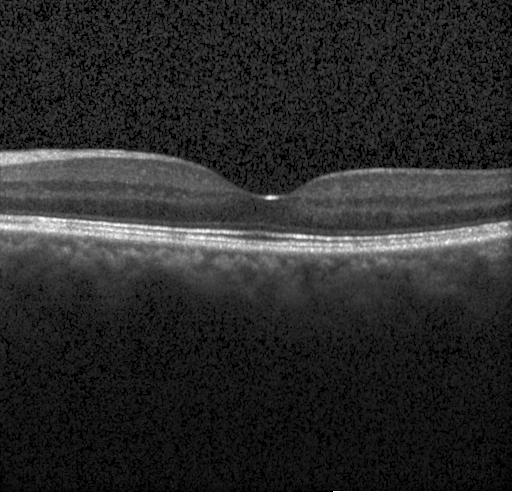 Horizontal scan through the fovea. Retinal OCT cross-section. Acquired on a Heidelberg Spectralis. Spectral-domain OCT — Macular OCT: no choroidal neovascularization, no diabetic macular edema, and no drusen.